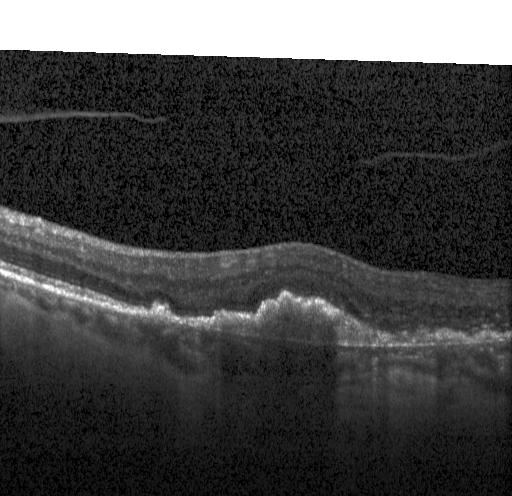 Diagnosis: CNV.